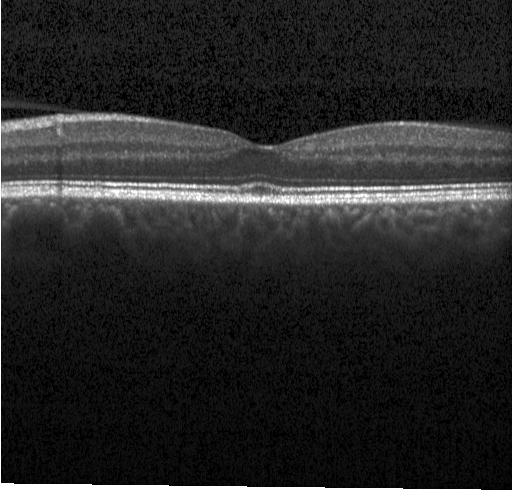

Optical coherence tomography B-scan, macular scan, instrument: Heidelberg Spectralis. Impression: no CNV, no DME, and no drusen.